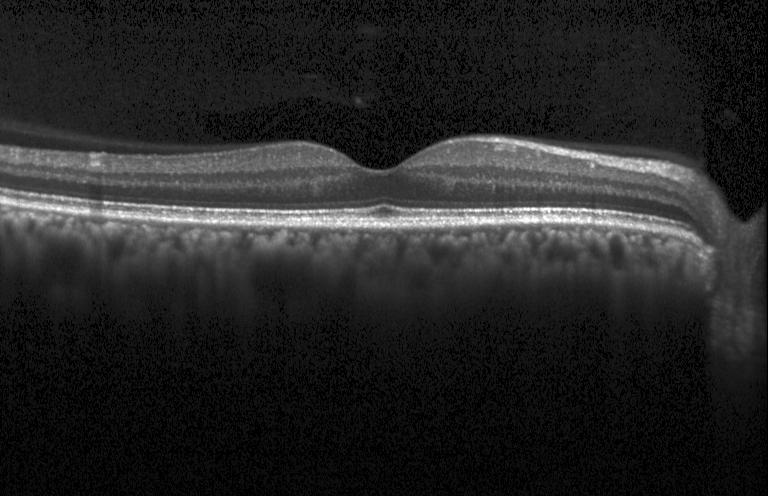
SD-OCT. OCT line scan. Instrument: Heidelberg Spectralis. Macular scan. This B-scan demonstrates no CNV, DME, or drusen.